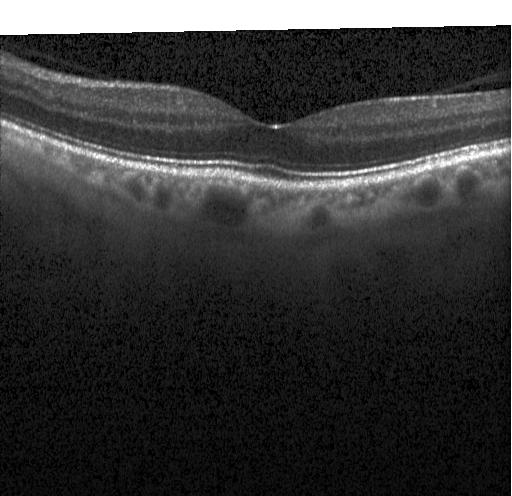 Retinal OCT B-scan · Heidelberg Spectralis · fovea-centered. Assessment: no evidence of choroidal neovascularization, diabetic macular edema, or drusen.